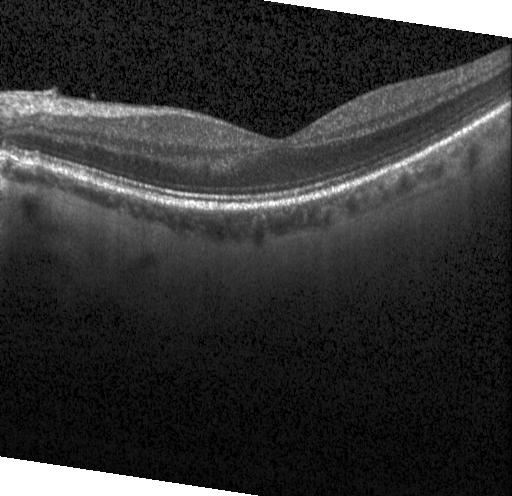

OCT B-scan. Heidelberg Spectralis — Finding: neither choroidal neovascularization, diabetic macular edema, nor drusen.